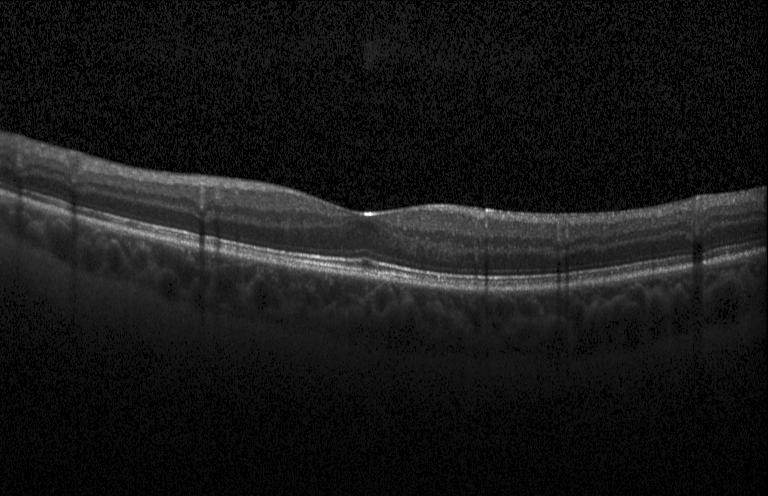

Retinal OCT B-scan — Diagnosis: no CNV, DME, or drusen.